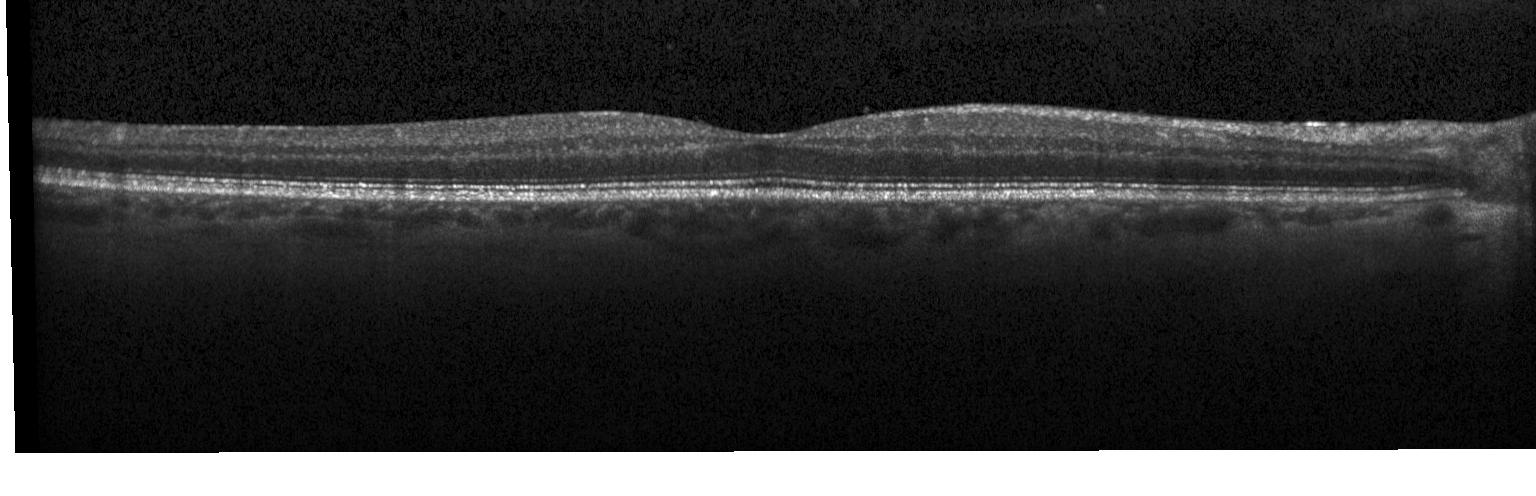
Optical coherence tomography scan · fovea-centered · SD-OCT. Finding: no evidence of CNV, DME, or drusen.